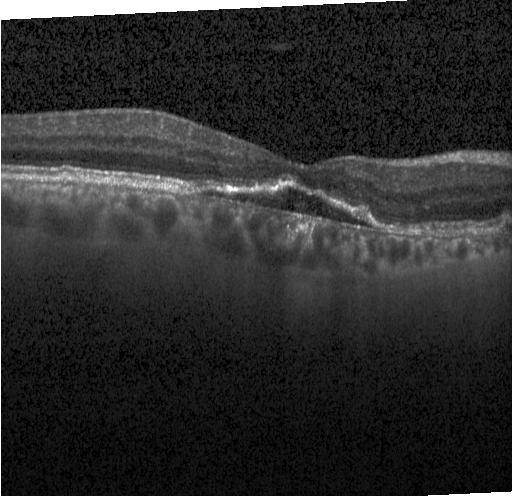

Macular scan. Acquired on a Heidelberg Spectralis. Spectral-domain OCT. Retinal OCT B-scan — Dx: a choroidal neovascular membrane.